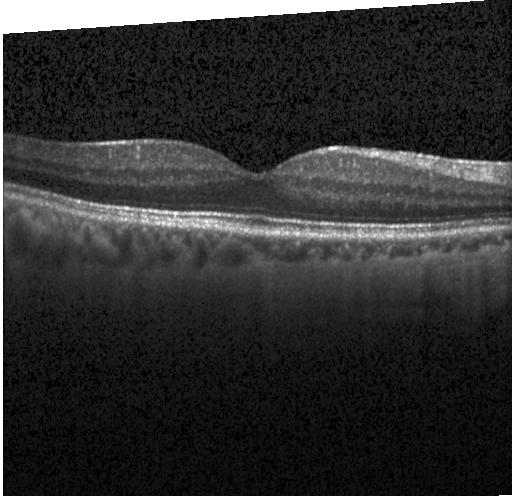

Finding: no choroidal neovascularization, no diabetic macular edema, and no drusen.